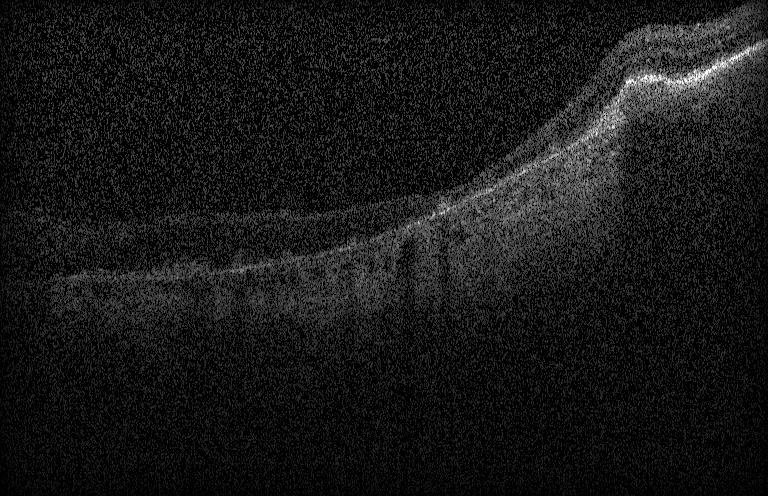

Horizontal scan through the fovea · spectral-domain OCT · OCT B-scan.
Impression: a choroidal neovascular membrane.